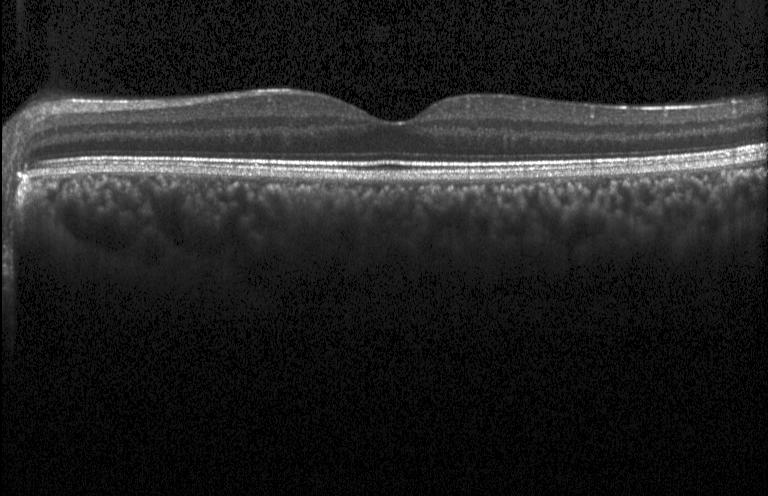
Spectral-domain OCT B-scan: no choroidal neovascularization, diabetic macular edema, or drusen.